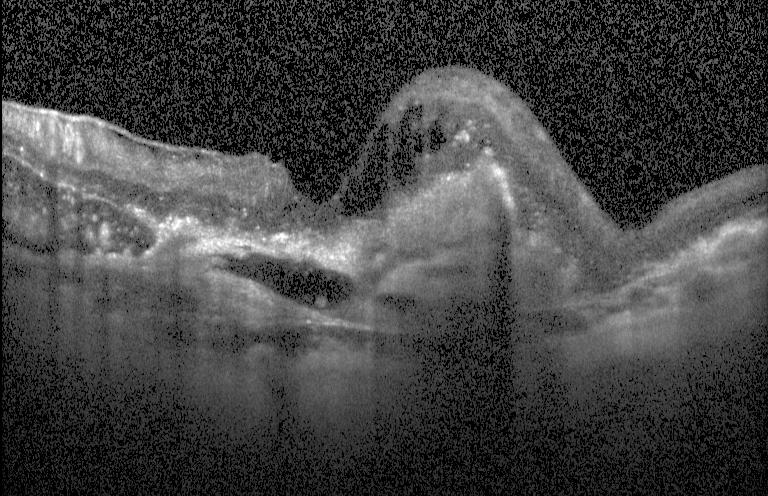 Impression: choroidal neovascularization.